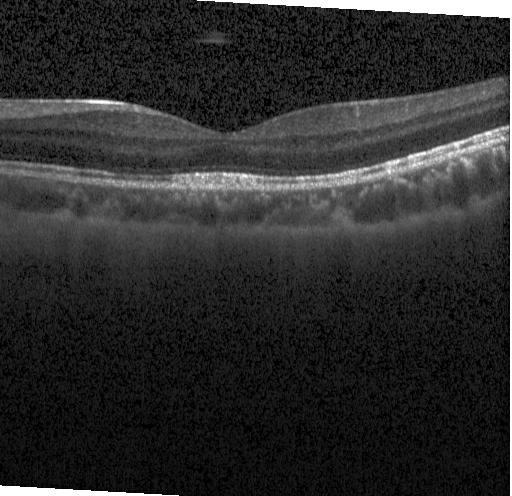
Optical coherence tomography scan · Heidelberg Spectralis OCT system.
Impression: no CNV, DME, or drusen.